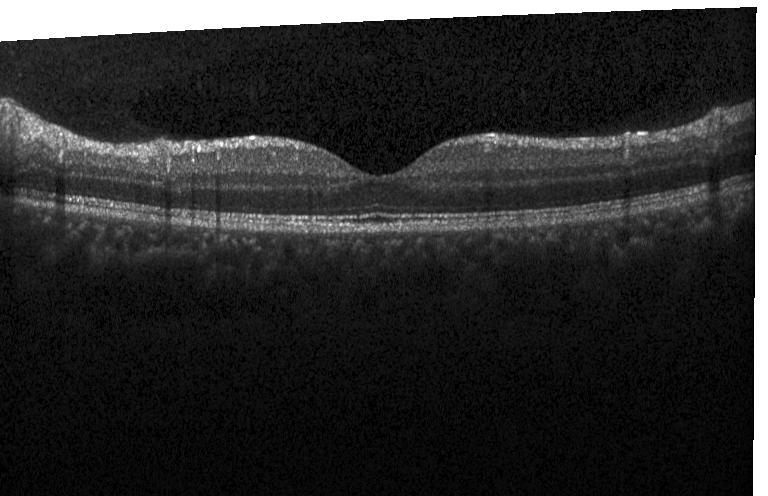 Impression: neither choroidal neovascularization, diabetic macular edema, nor drusen.